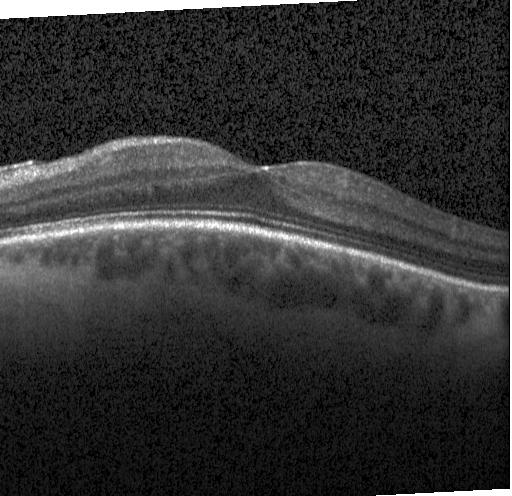
Horizontal scan through the fovea; optical coherence tomography scan; Heidelberg Spectralis — Assessment: no evidence of CNV, DME, or drusen.